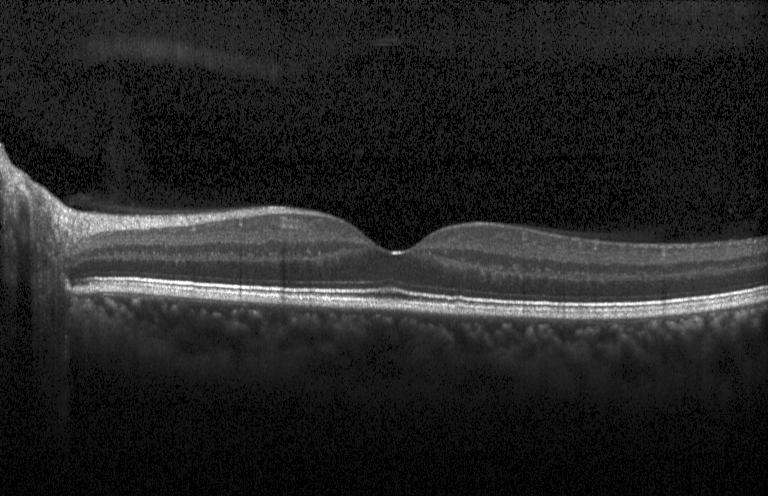 Heidelberg Spectralis OCT system · retinal OCT cross-section — Diagnosis: no evidence of choroidal neovascularization, diabetic macular edema, or drusen.